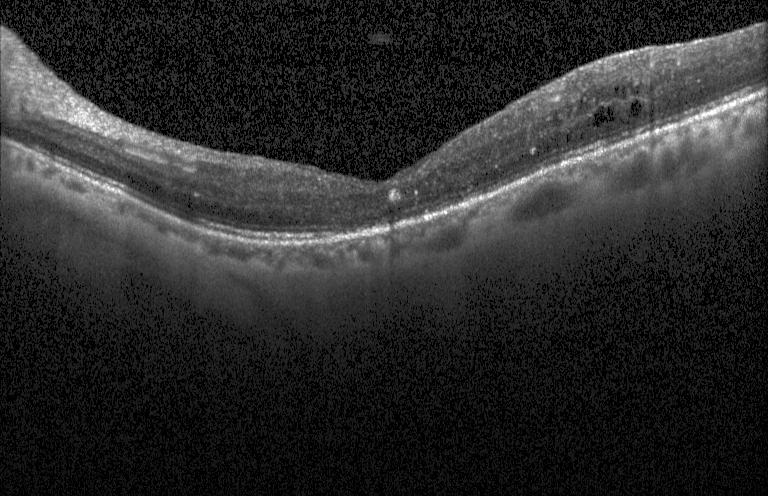

OCT scan showing DME.